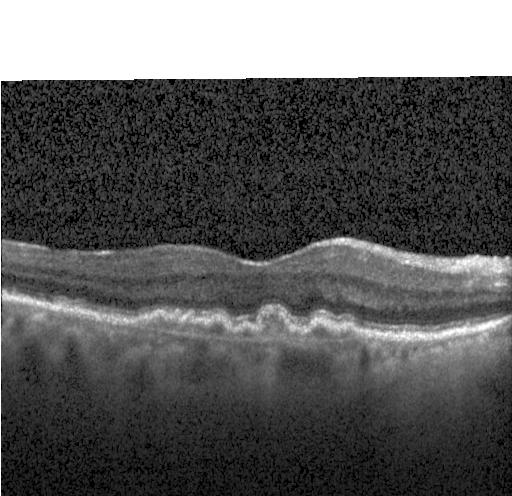 Choroidal neovascularization.